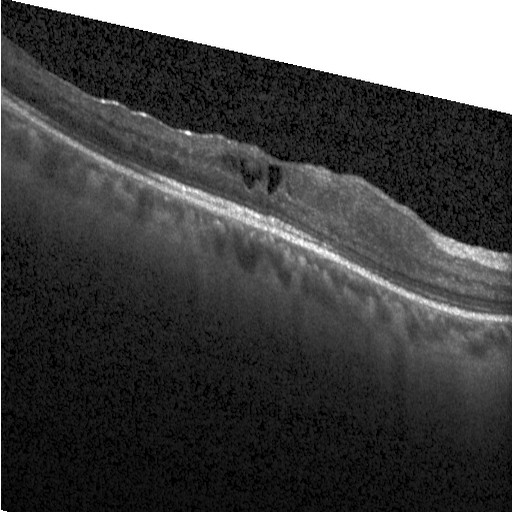

Spectral-domain optical coherence tomography, Heidelberg Spectralis OCT system, retinal OCT cross-section, macular scan.
Impression: diabetic macular edema (DME).